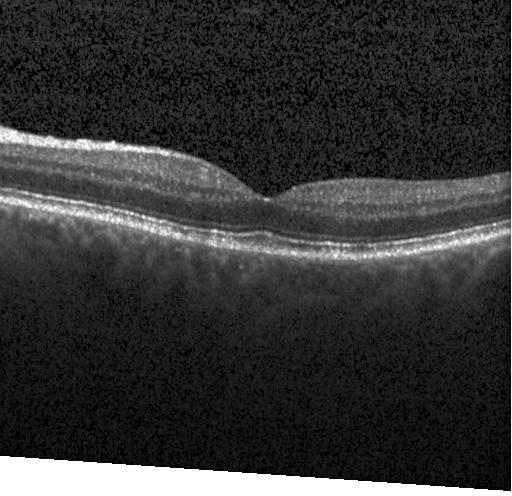 Optical coherence tomography scan.
Diagnosis: no CNV, no DME, and no drusen.